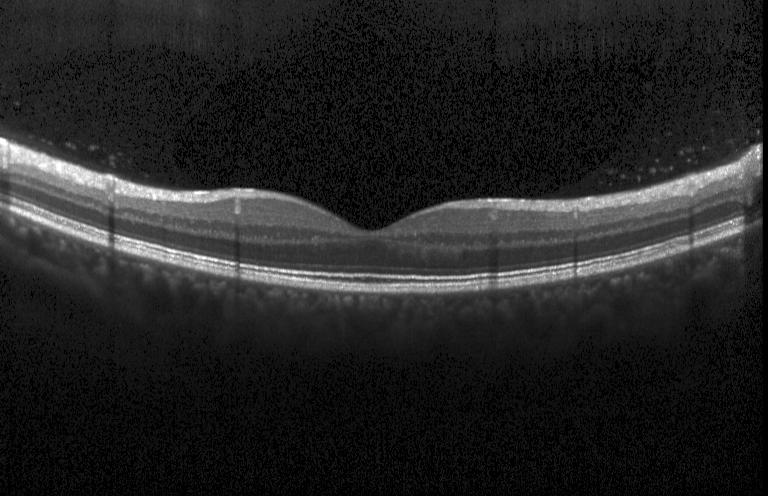

Optical coherence tomography B-scan; Heidelberg Spectralis; through the macula — Impression: no evidence of choroidal neovascularization, diabetic macular edema, or drusen.